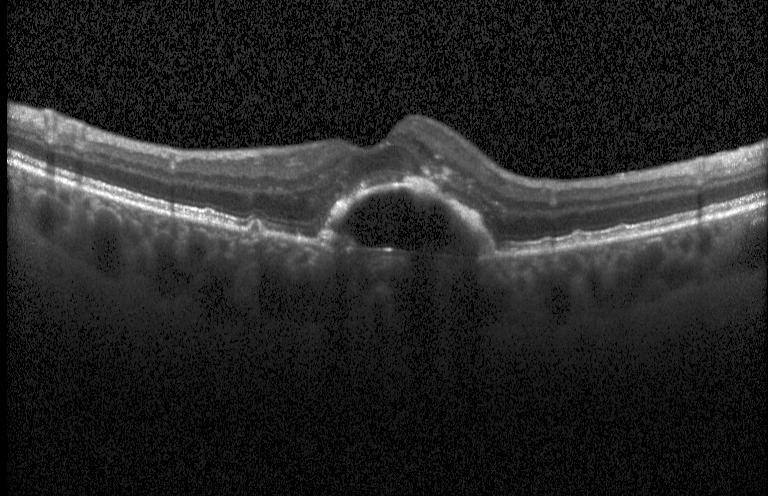 Spectral-domain optical coherence tomography. Retinal OCT B-scan. This B-scan demonstrates choroidal neovascularization (CNV).